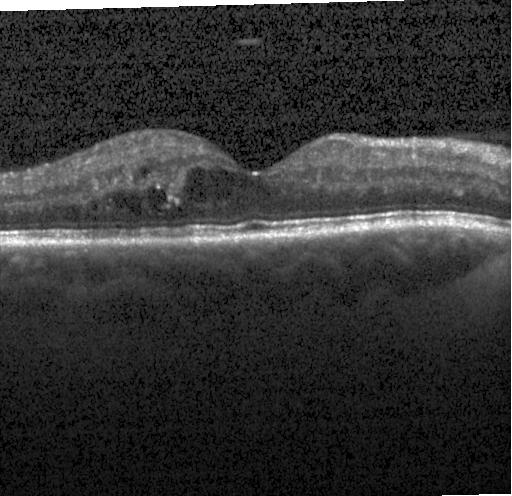
Optical coherence tomography B-scan, macular scan — Finding: DME.